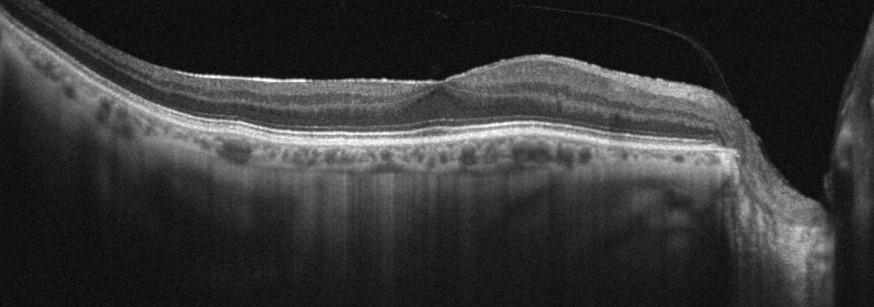 Instrument: Optovue Avanti RTVue XR, OCT B-scan. Finding: no evidence of AMD, DME, ERM, RAO, RVO, or VID.